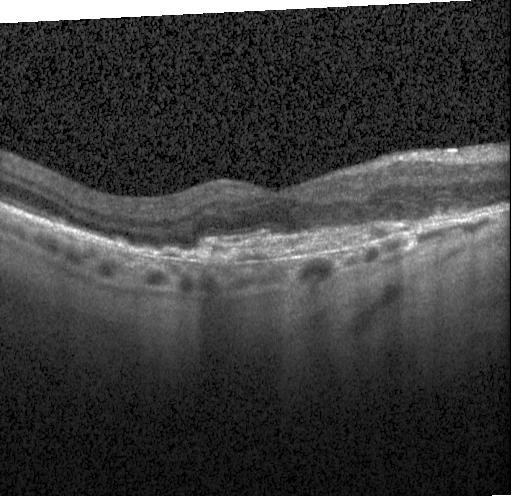 Optical coherence tomography B-scan · Heidelberg Spectralis OCT system
Finding: choroidal neovascularization (CNV).